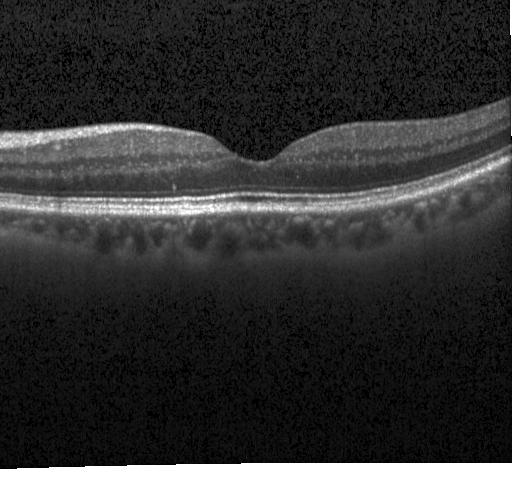 OCT line scan. No choroidal neovascularization, no diabetic macular edema, and no drusen.